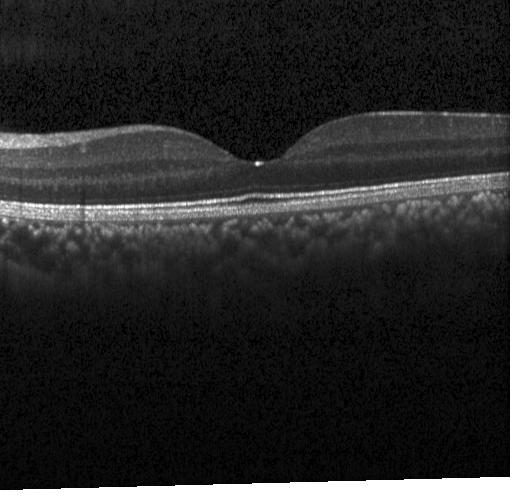
OCT line scan. SD-OCT
Impression: neither CNV, DME, nor drusen.